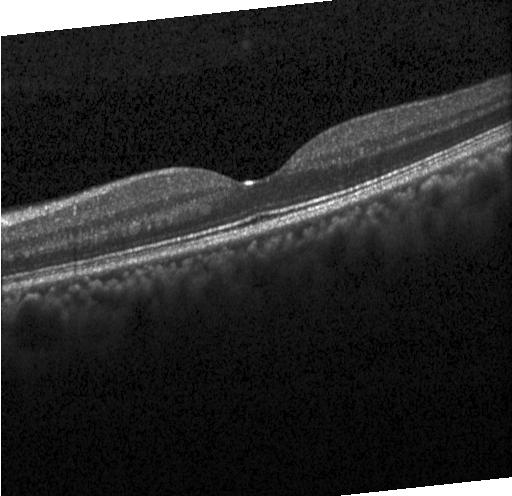

Instrument: Heidelberg Spectralis; optical coherence tomography scan
Impression: no choroidal neovascularization, no diabetic macular edema, and no drusen.